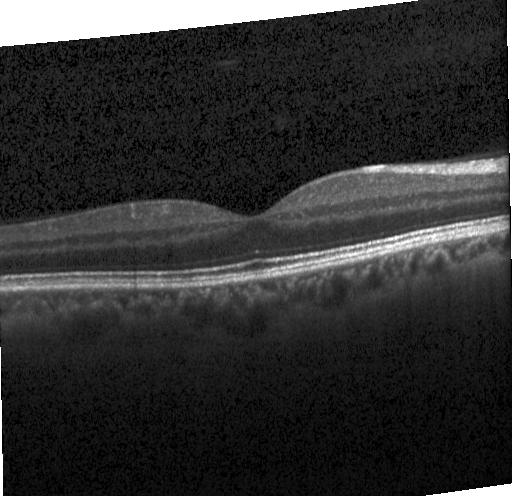

Heidelberg Spectralis OCT system; spectral-domain OCT; through the macula; retinal OCT cross-section — This B-scan demonstrates no CNV, no DME, and no drusen.